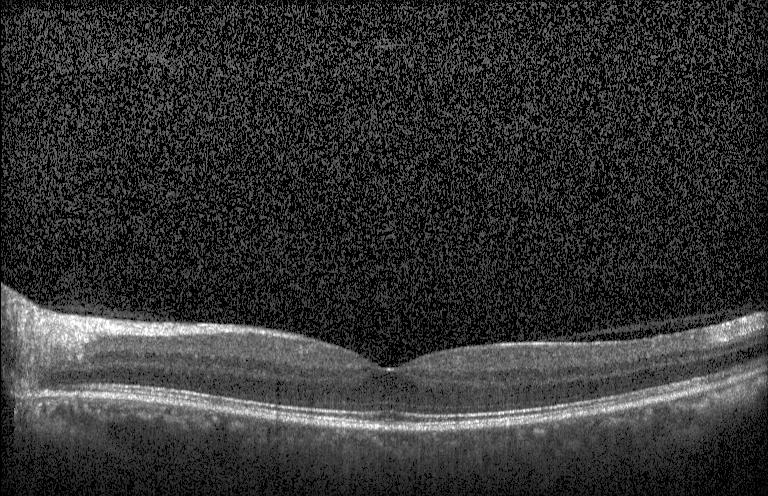

Acquired on a Heidelberg Spectralis · macular scan · OCT line scan. Macular OCT: neither CNV, DME, nor drusen.